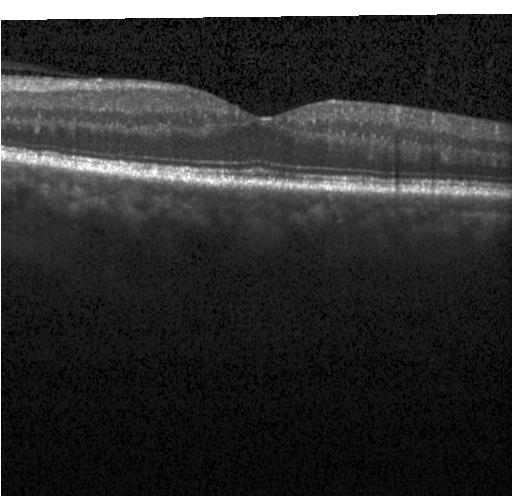

Finding: no evidence of CNV, DME, or drusen.